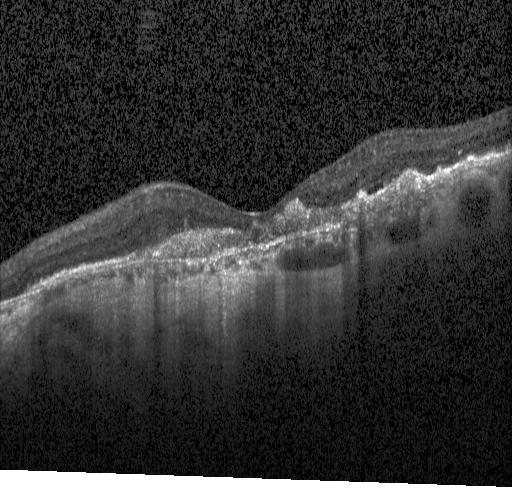 Acquired on a Heidelberg Spectralis · OCT line scan · SD-OCT — A choroidal neovascular membrane.